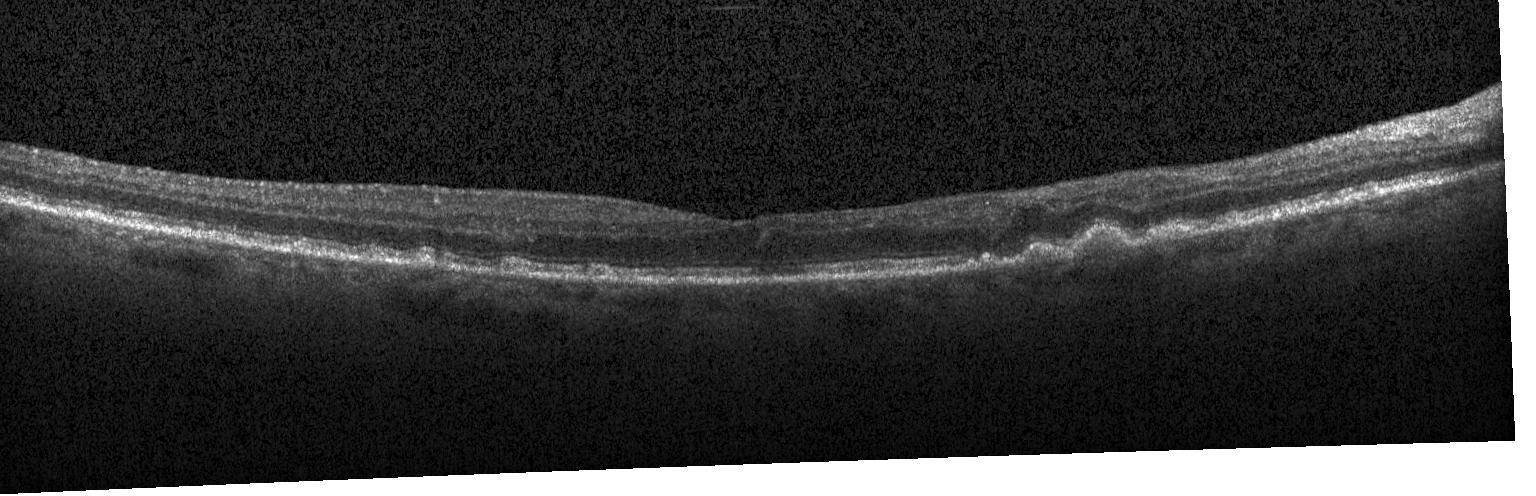
SD-OCT; OCT line scan.
Macular OCT: drusen.